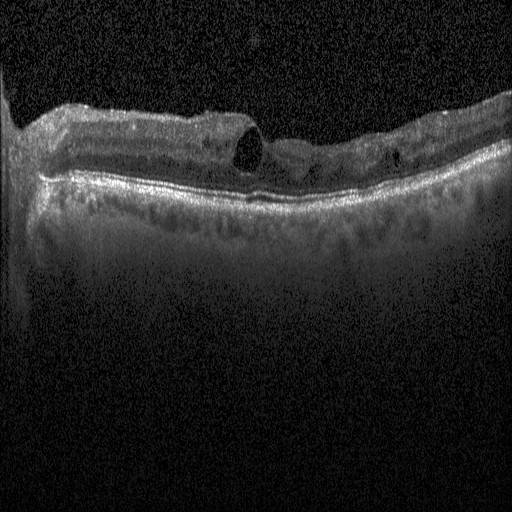

OCT scan showing diabetic macular edema (DME).